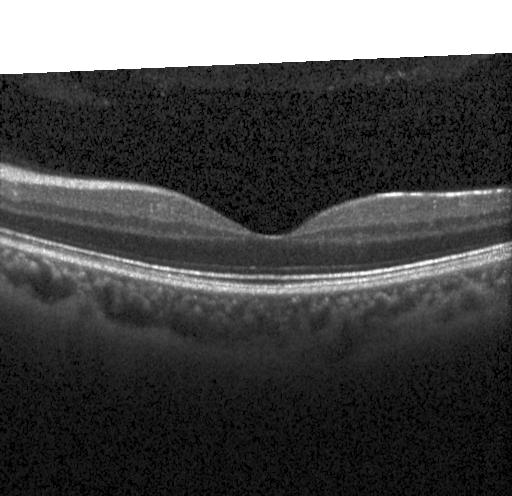

Macular OCT: neither CNV, DME, nor drusen.